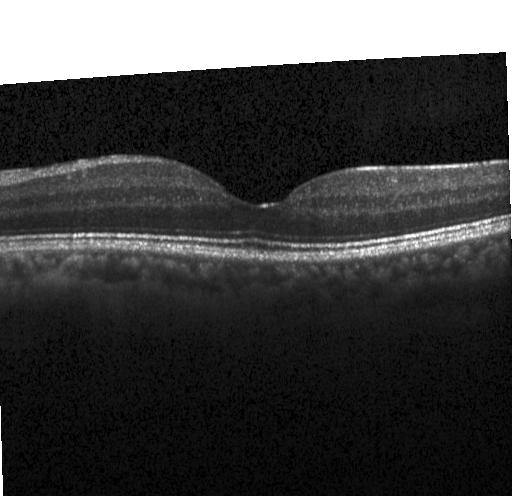

Diagnosis: no evidence of CNV, DME, or drusen.